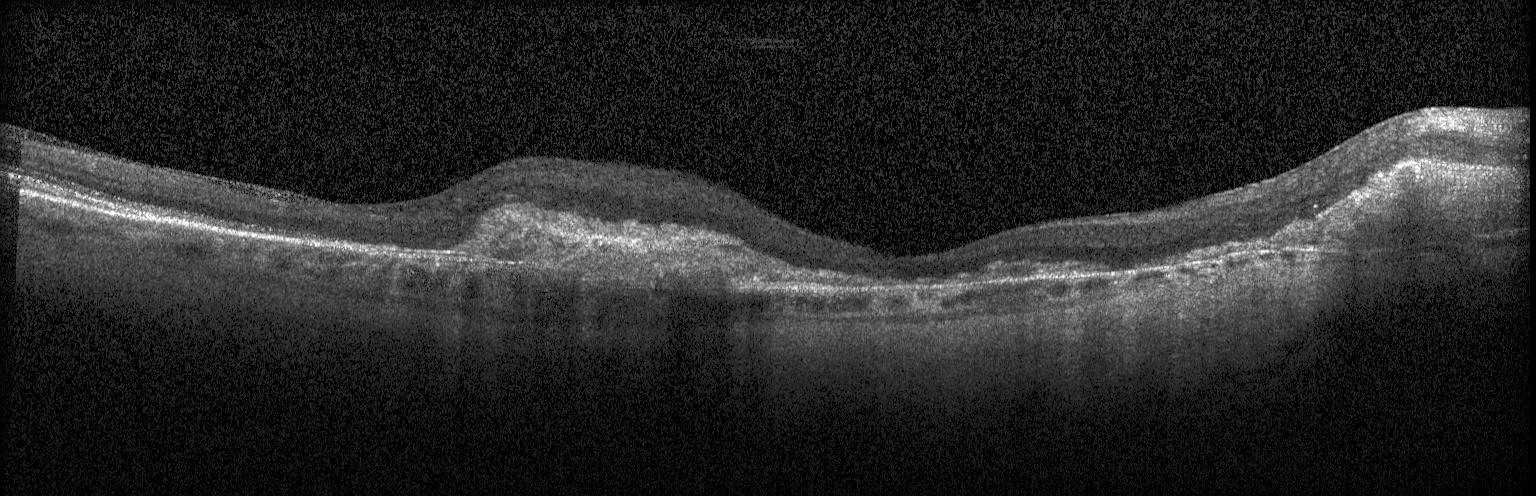
Spectral-domain OCT B-scan: a choroidal neovascular membrane.